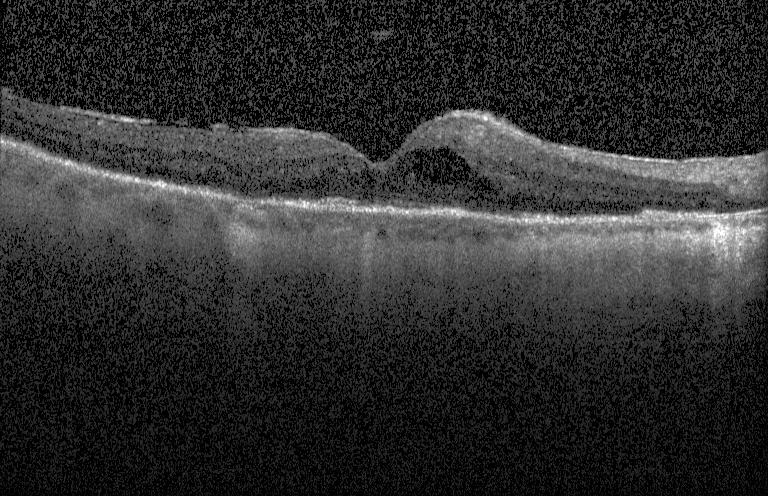

Impression: diabetic macular edema (DME).